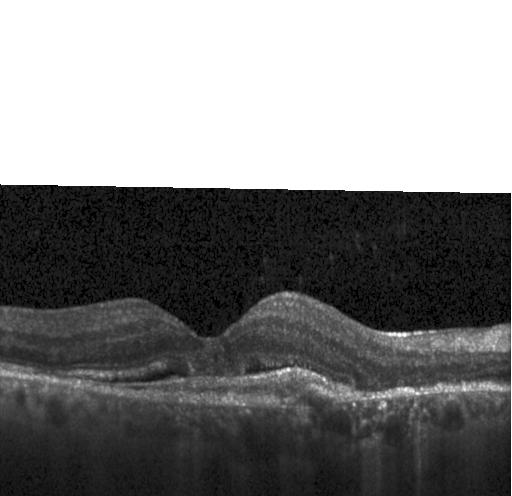

Instrument: Heidelberg Spectralis. Retinal OCT B-scan. Finding: a choroidal neovascular membrane.